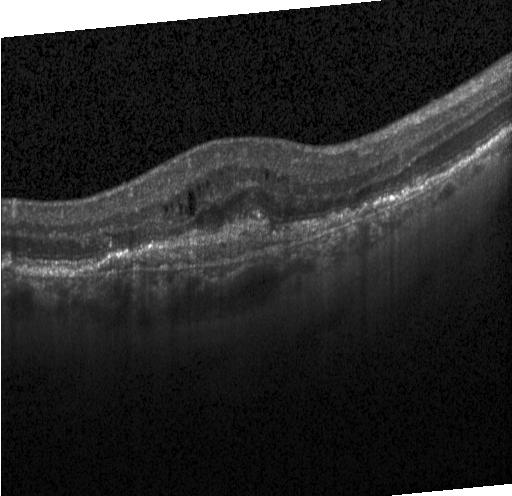

Optical coherence tomography scan
Finding: choroidal neovascularization.